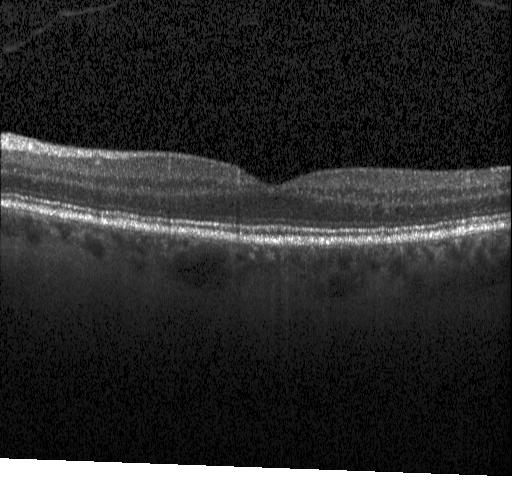
No choroidal neovascularization, diabetic macular edema, or drusen.